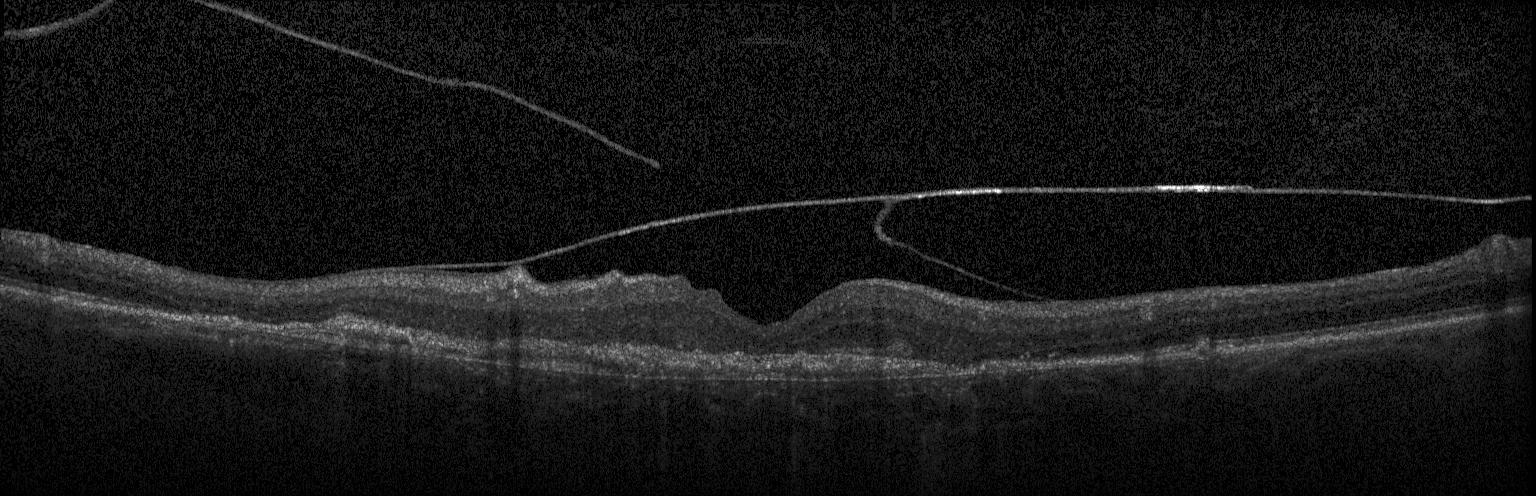 Spectral-domain optical coherence tomography; Heidelberg Spectralis OCT system; retinal OCT B-scan — The scan shows a choroidal neovascular membrane.